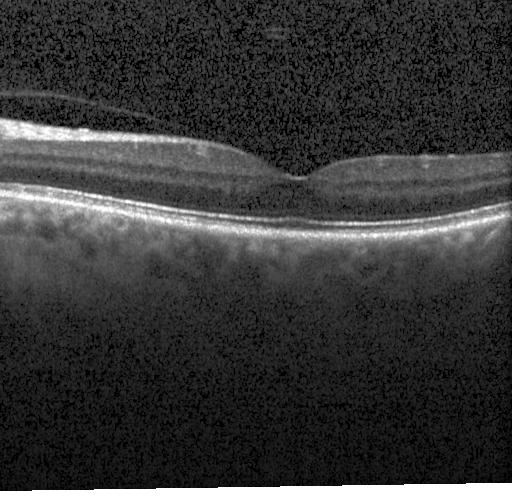 Through the macula. Spectral-domain OCT. OCT line scan.
The scan shows neither choroidal neovascularization, diabetic macular edema, nor drusen.